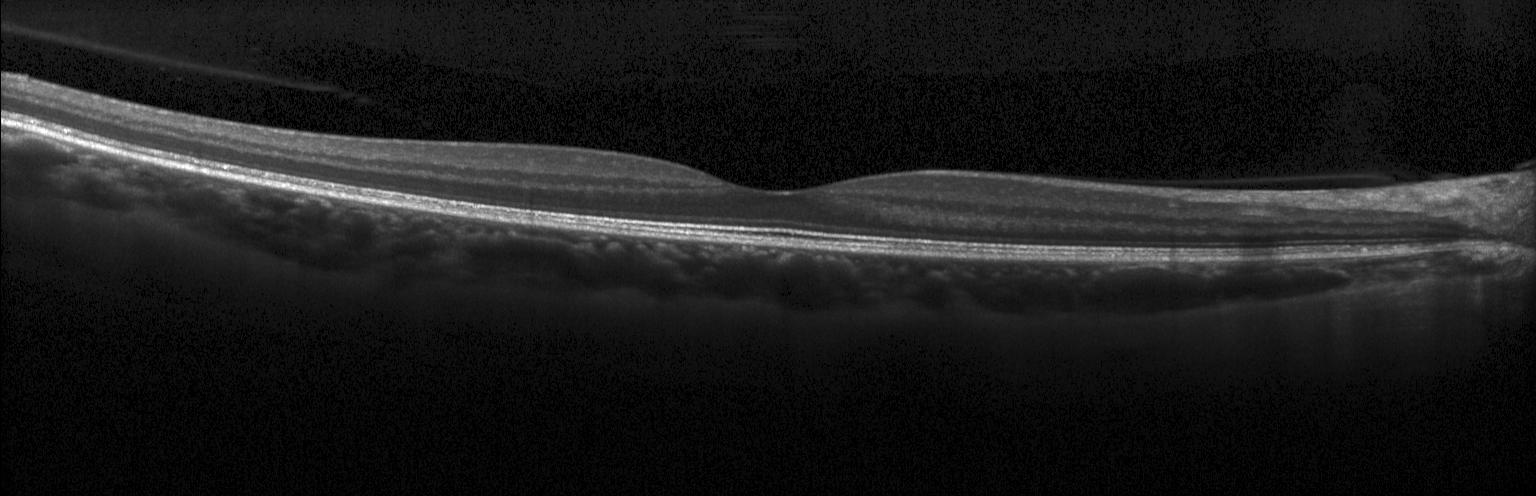

This B-scan demonstrates no CNV, no DME, and no drusen.